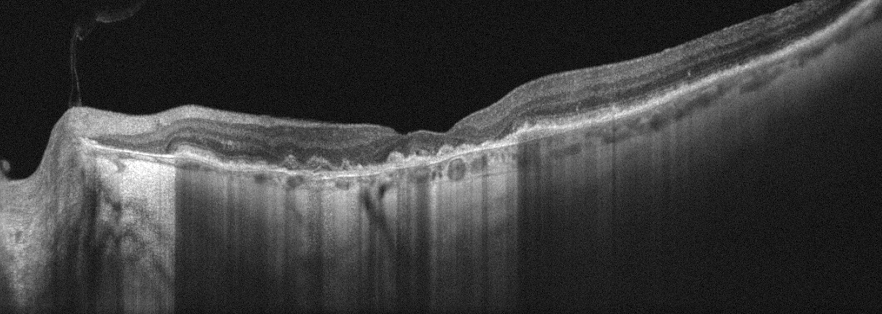
Left eye. OCT B-scan. Assessment: age-related macular degeneration.